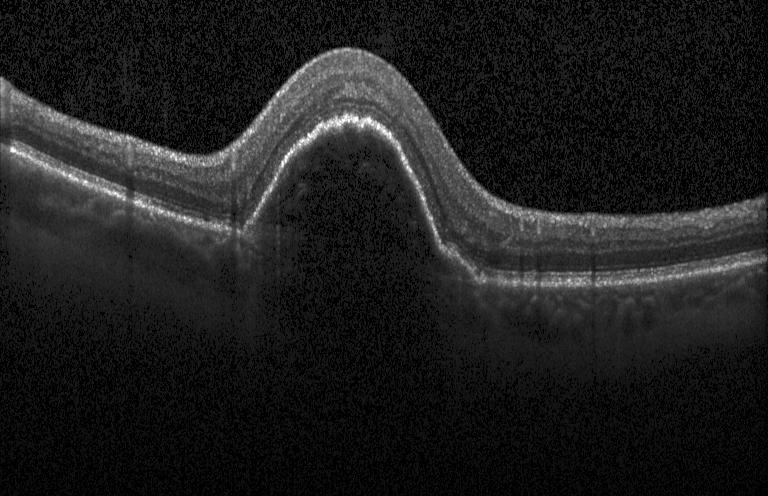
OCT B-scan, Heidelberg Spectralis OCT system, fovea-centered. Dx: a choroidal neovascular membrane.